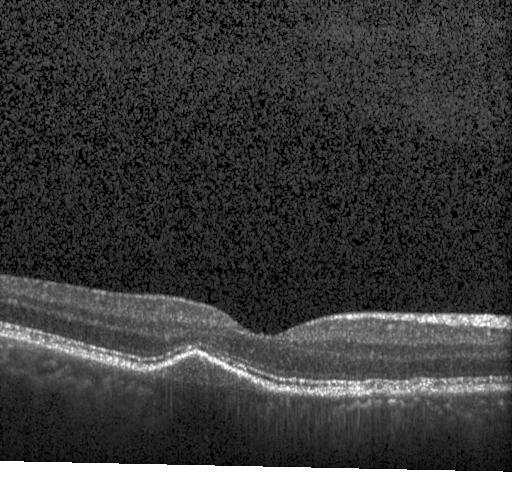 The scan shows multiple drusen.